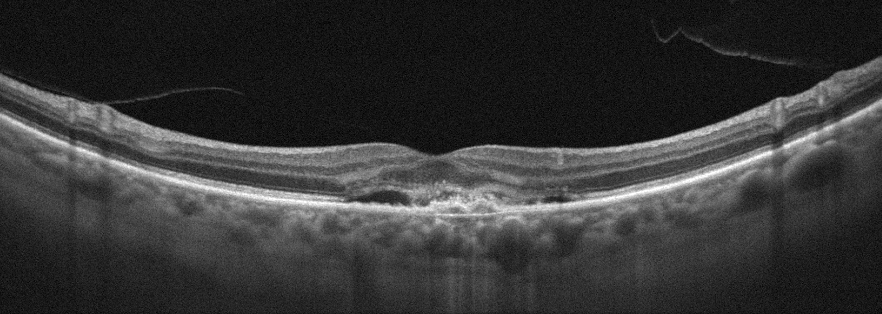

Oculus dexter, optical coherence tomography B-scan. Finding: AMD.